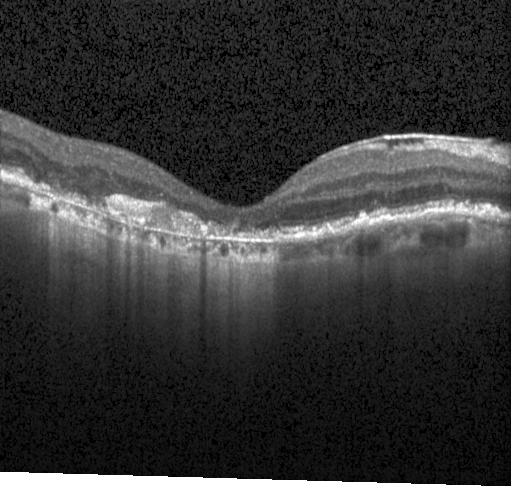 OCT line scan.
Choroidal neovascularization.